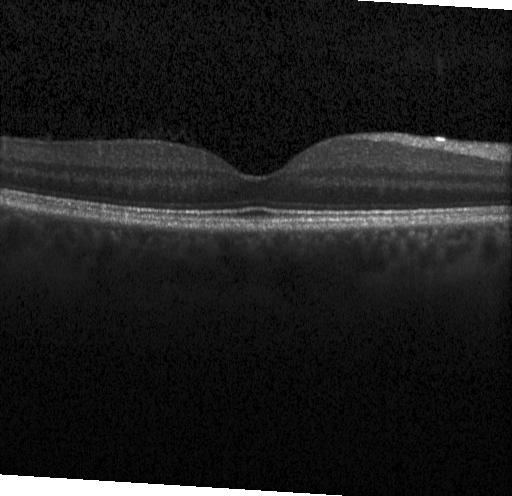
Optical coherence tomography scan, acquired on a Heidelberg Spectralis, spectral-domain optical coherence tomography, centered on the fovea.
Dx: no CNV, DME, or drusen.